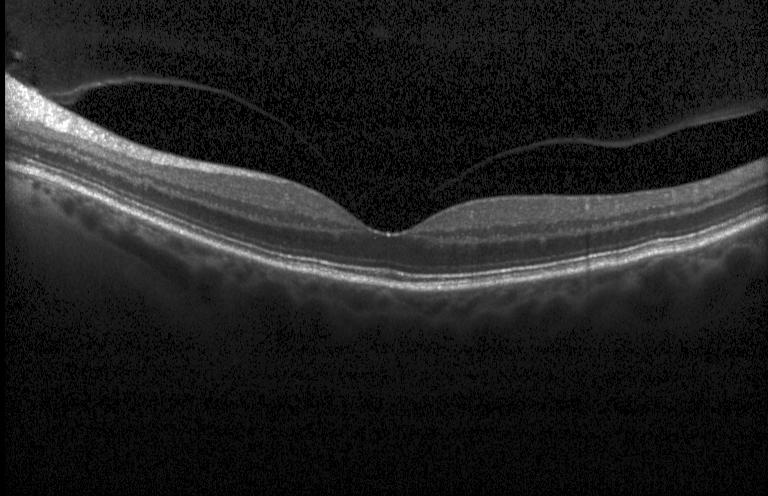
Optical coherence tomography B-scan.
This B-scan demonstrates no evidence of CNV, DME, or drusen.